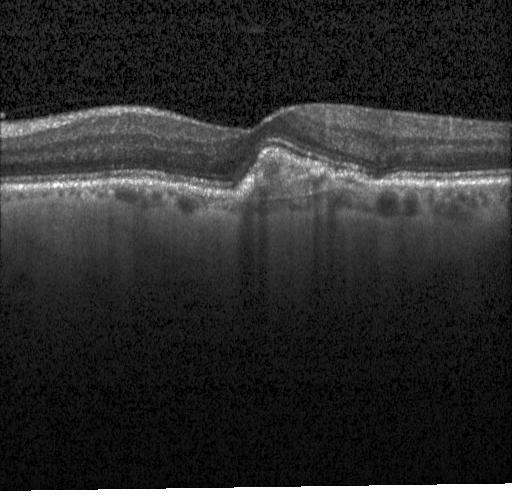

OCT line scan.
Impression: CNV.